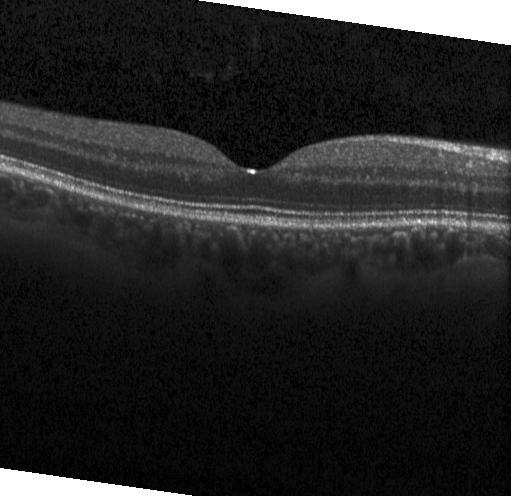
Through the macula, optical coherence tomography scan
The scan shows no evidence of choroidal neovascularization, diabetic macular edema, or drusen.